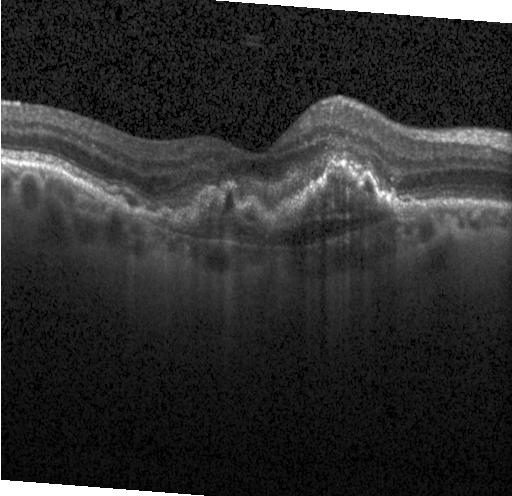
Heidelberg Spectralis; optical coherence tomography scan; fovea-centered; SD-OCT. Choroidal neovascularization.